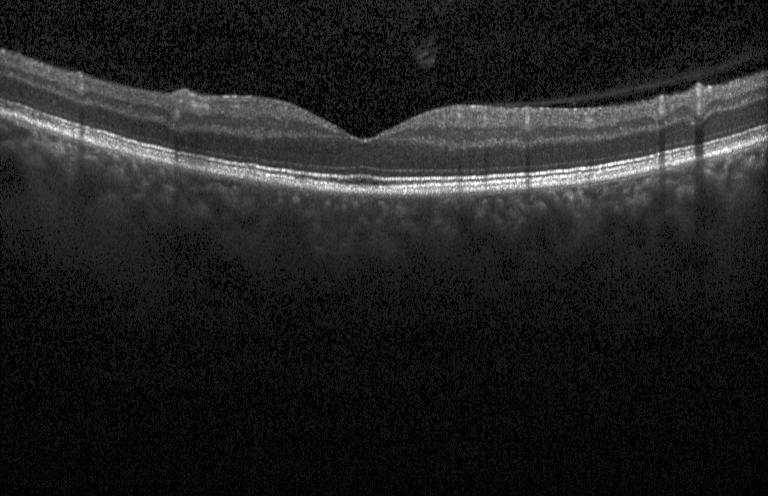
Finding: neither choroidal neovascularization, diabetic macular edema, nor drusen.